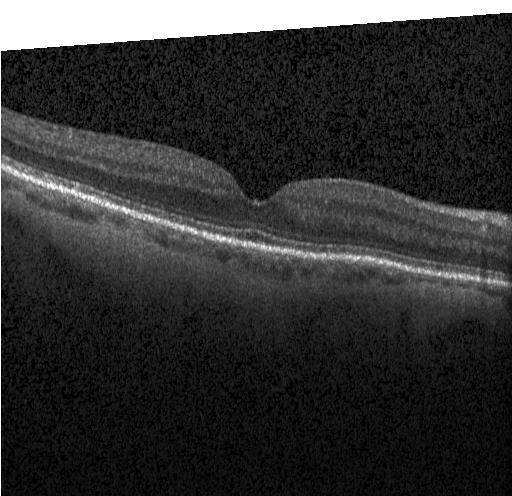 Retinal OCT cross-section; Heidelberg Spectralis; centered on the fovea. This B-scan demonstrates no evidence of CNV, DME, or drusen.